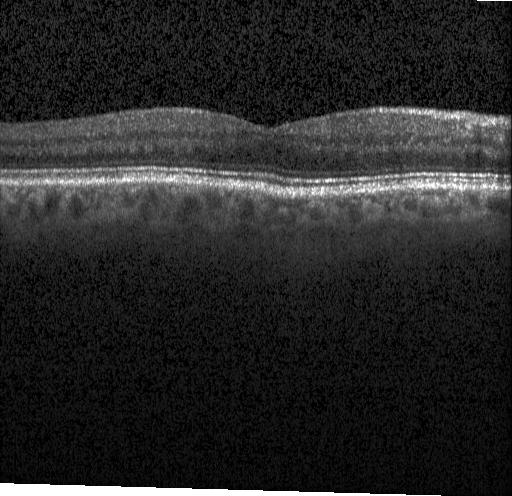
OCT line scan
This B-scan demonstrates no choroidal neovascularization, diabetic macular edema, or drusen.